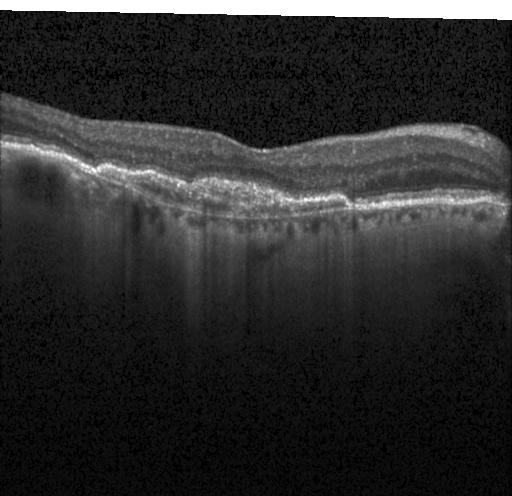 Dx: choroidal neovascularization (CNV).